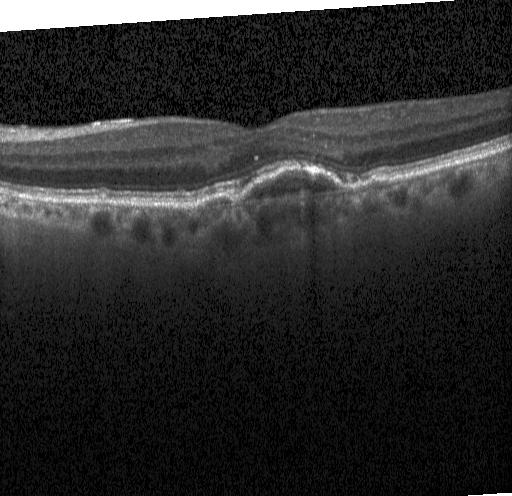 Optical coherence tomography scan
Diagnosis: choroidal neovascularization.